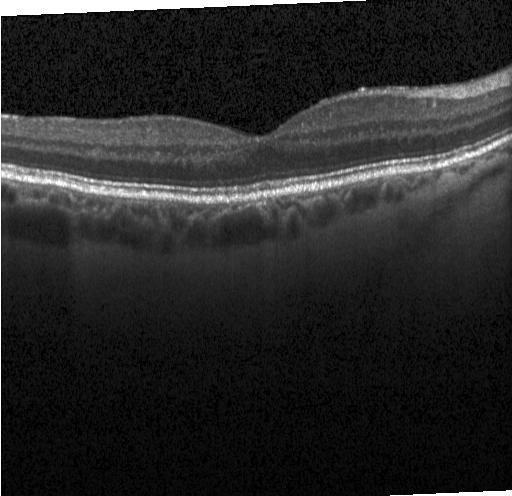

Optical coherence tomography B-scan · SD-OCT
Finding: no choroidal neovascularization, diabetic macular edema, or drusen.